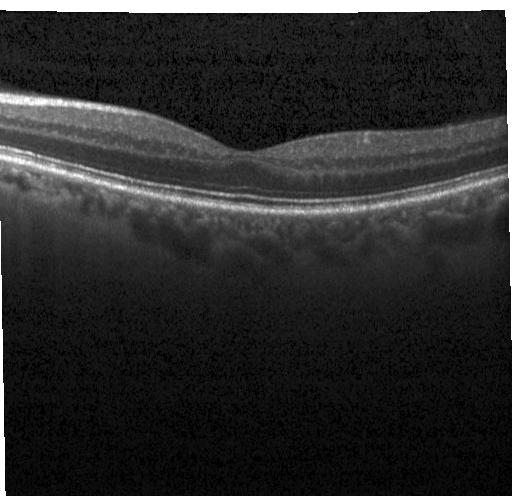 OCT line scan
Dx: no choroidal neovascularization, no diabetic macular edema, and no drusen.